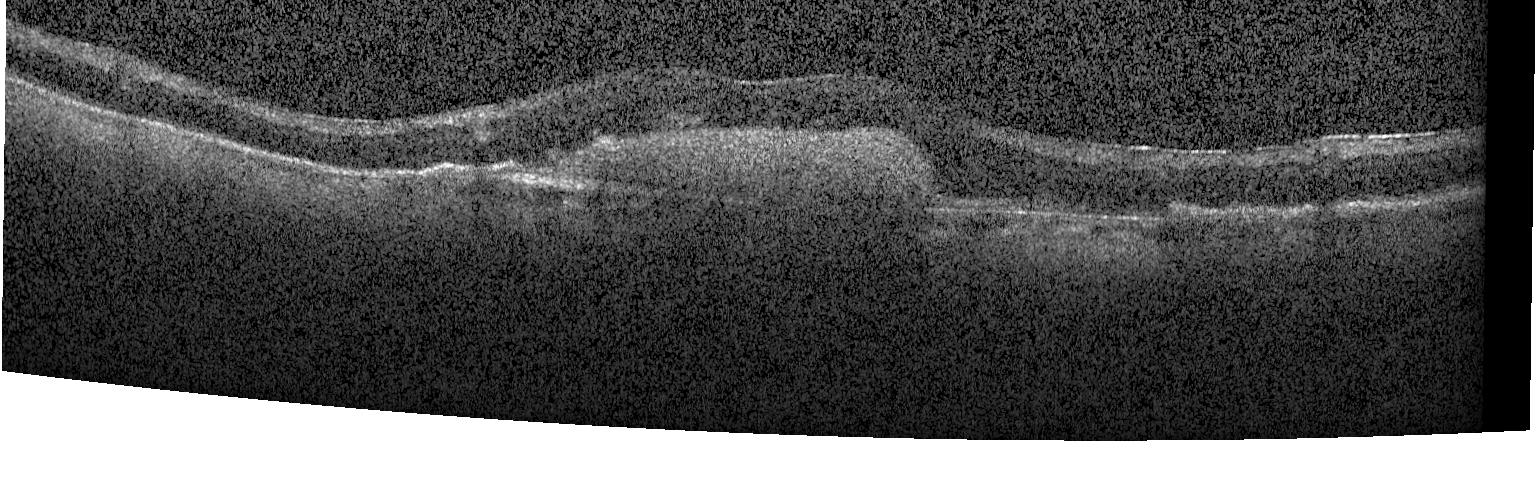

Finding: a choroidal neovascular membrane.